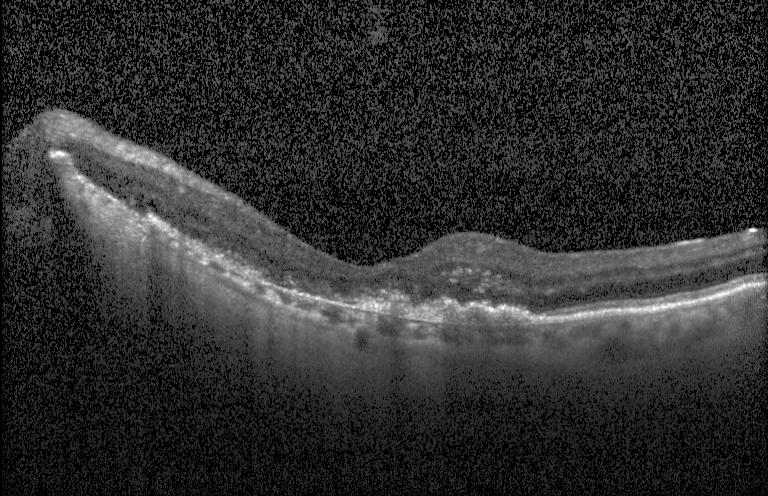

Retinal OCT B-scan
OCT finding: CNV.